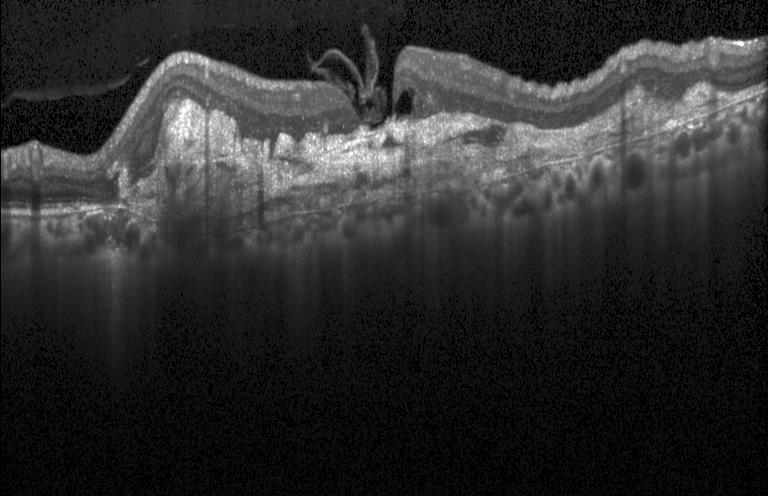
Optical coherence tomography scan — Finding: a choroidal neovascular membrane.